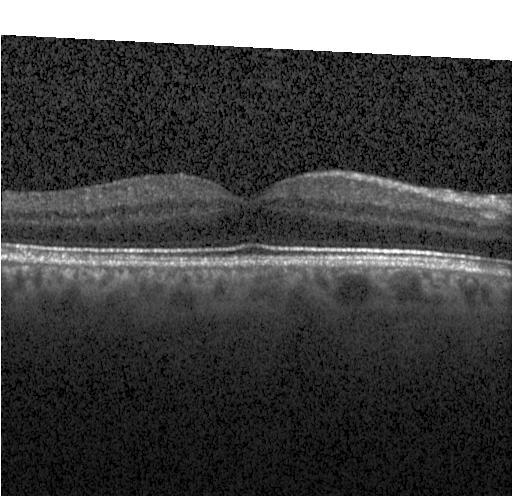

No choroidal neovascularization, no diabetic macular edema, and no drusen.